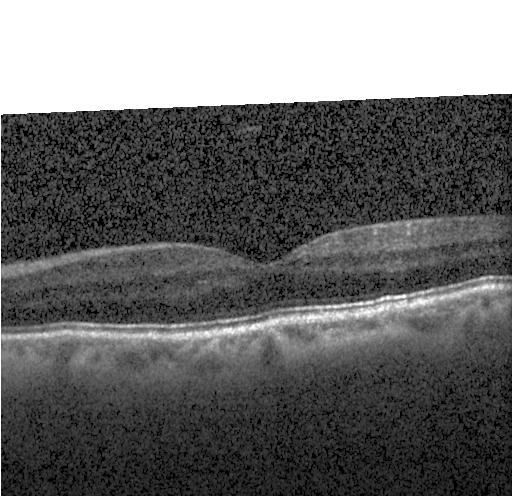 Fovea-centered; optical coherence tomography scan. Diagnosis: no CNV, DME, or drusen.